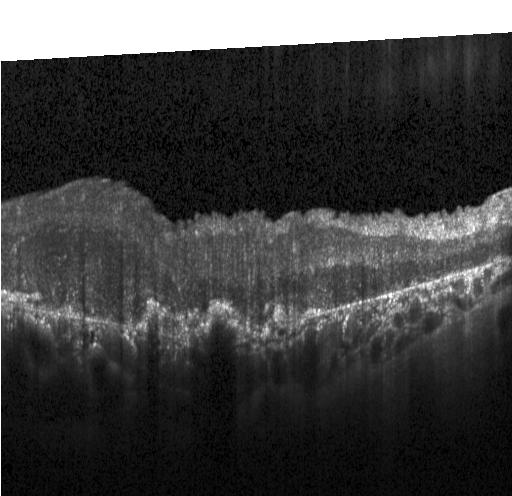
Optical coherence tomography B-scan. The scan shows a choroidal neovascular membrane.